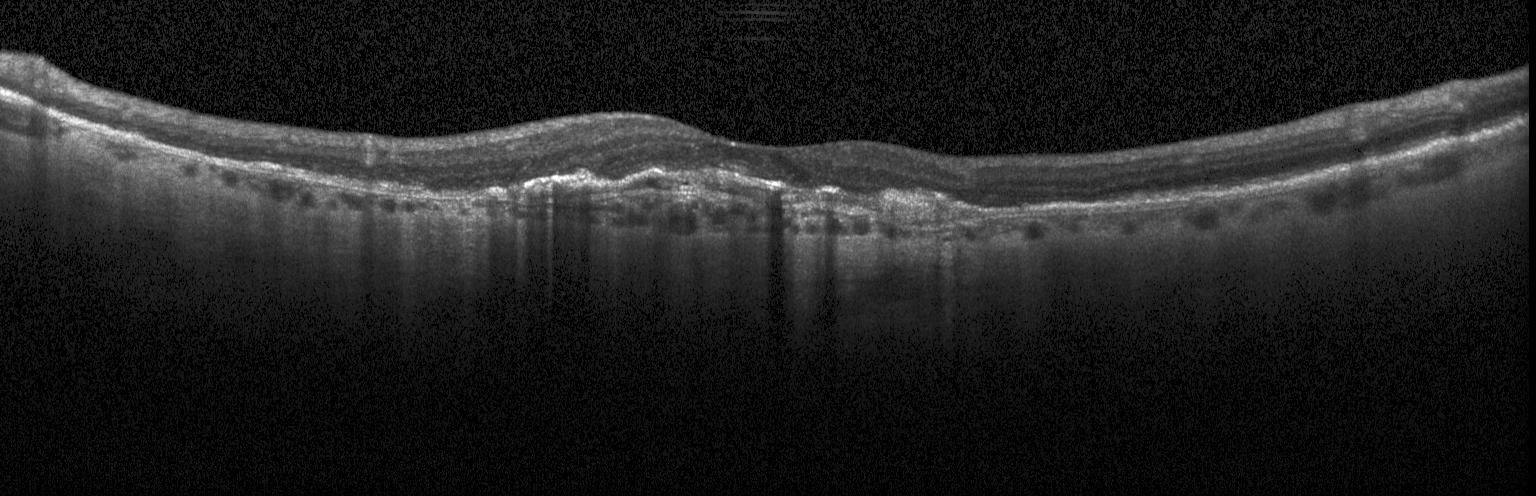

OCT finding: a choroidal neovascular membrane.